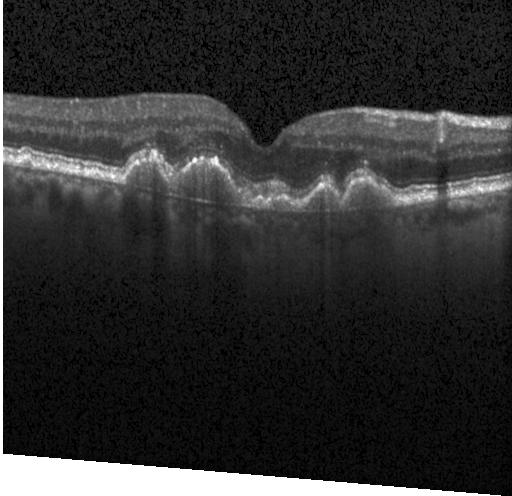 Retinal OCT B-scan, SD-OCT, Heidelberg Spectralis OCT system — Finding: drusen.